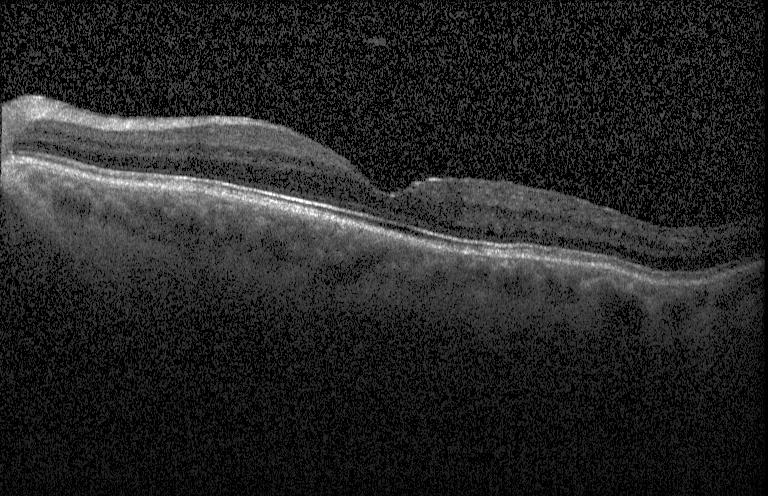 Macular OCT: no choroidal neovascularization, diabetic macular edema, or drusen.